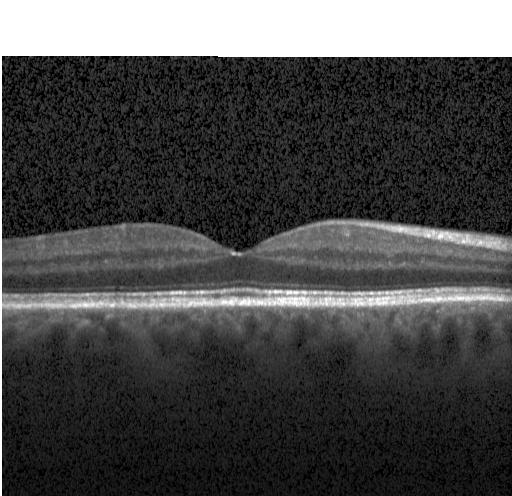 Dx: no CNV, no DME, and no drusen.